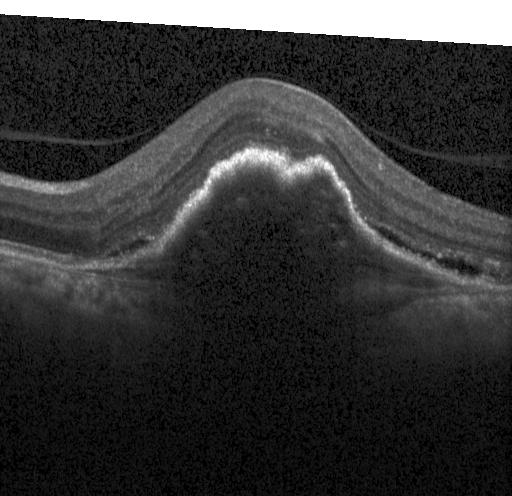 Dx: choroidal neovascularization.